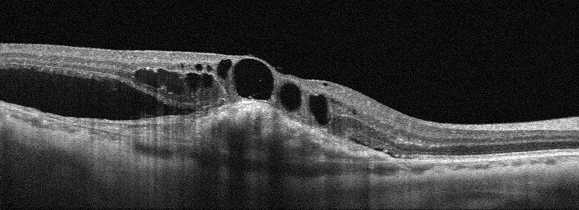

Right eye; OCT B-scan. Macular OCT: AMD.